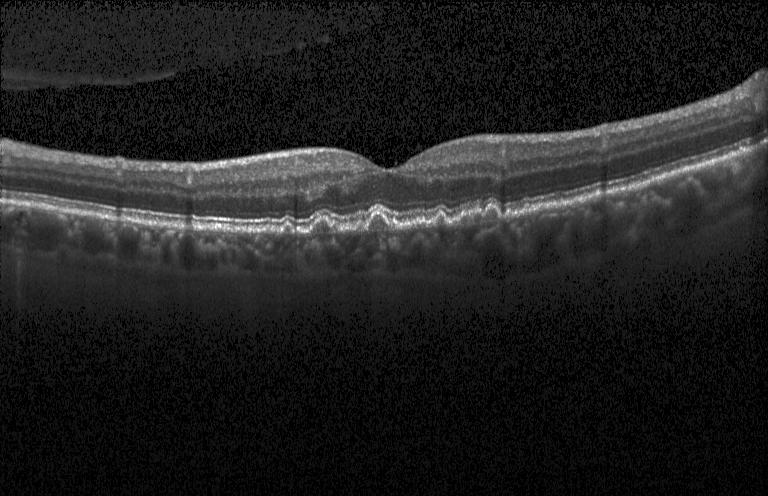 Heidelberg Spectralis. Retinal OCT B-scan. Horizontal scan through the fovea. Diagnosis: multiple drusen.